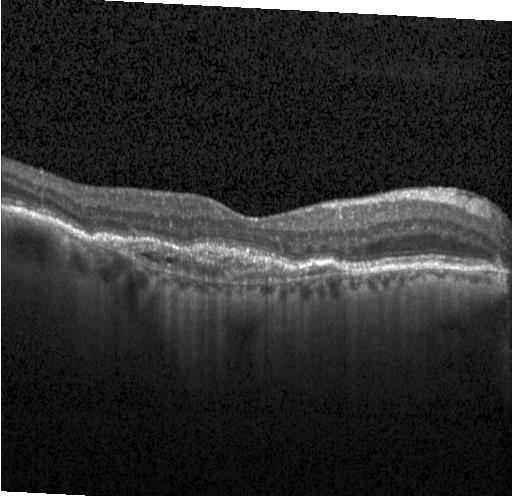
Finding: choroidal neovascularization (CNV).